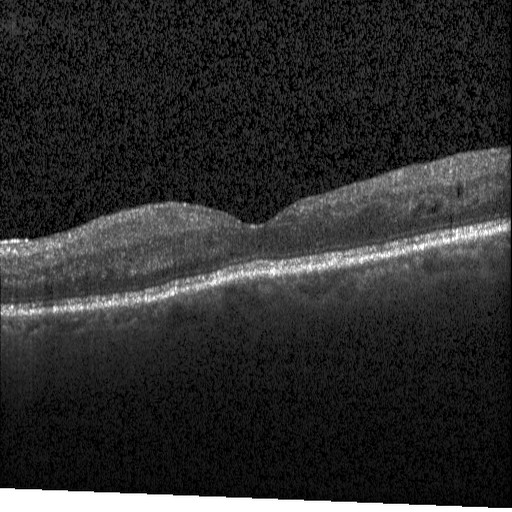
Dx: DME.